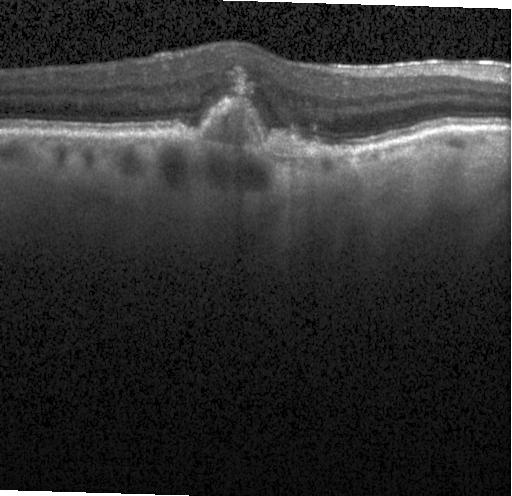 Spectral-domain optical coherence tomography; macular scan; acquired on a Heidelberg Spectralis; retinal OCT B-scan
Dx: choroidal neovascularization.